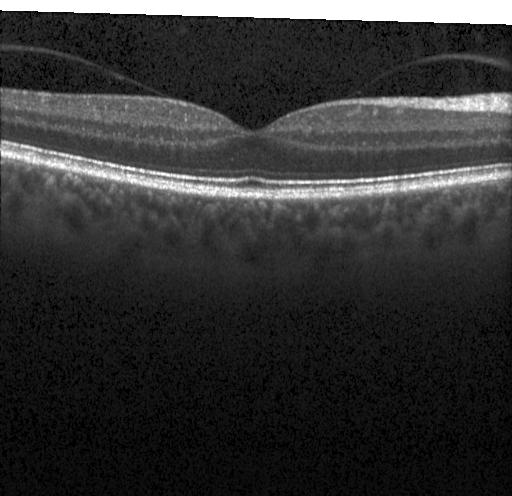
No evidence of choroidal neovascularization, diabetic macular edema, or drusen.